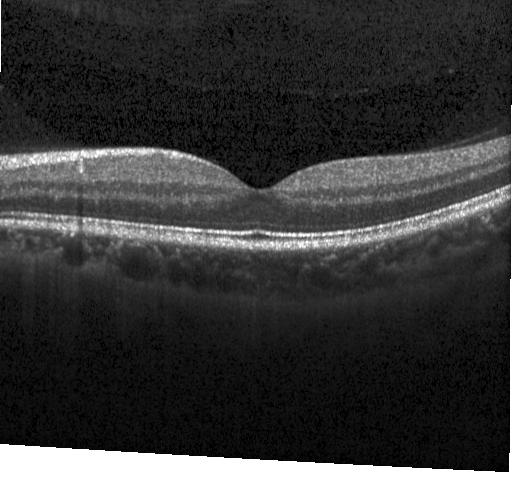
Instrument: Heidelberg Spectralis · macular scan · spectral-domain optical coherence tomography · optical coherence tomography scan.
This B-scan demonstrates no evidence of choroidal neovascularization, diabetic macular edema, or drusen.